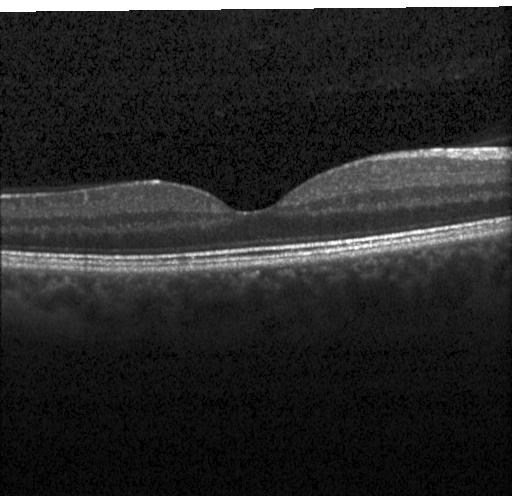 Finding: no evidence of CNV, DME, or drusen.